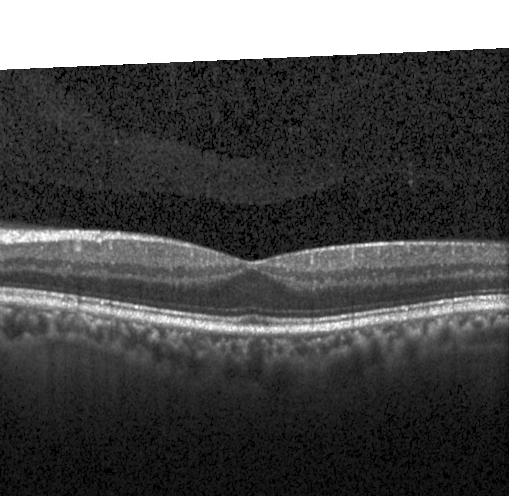
This B-scan demonstrates no choroidal neovascularization, no diabetic macular edema, and no drusen.